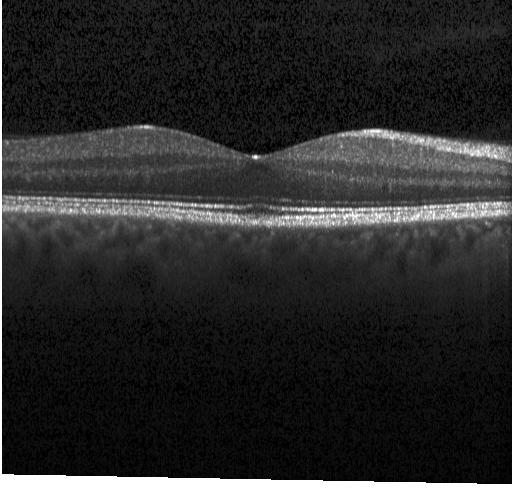
Diagnosis: no evidence of CNV, DME, or drusen.